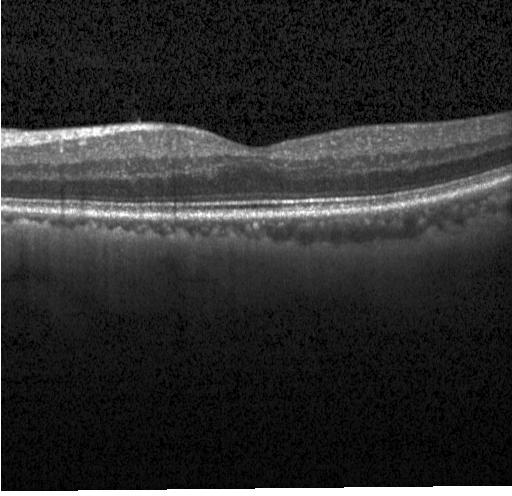 Centered on the fovea, spectral-domain optical coherence tomography, optical coherence tomography scan
Assessment: no choroidal neovascularization, diabetic macular edema, or drusen.